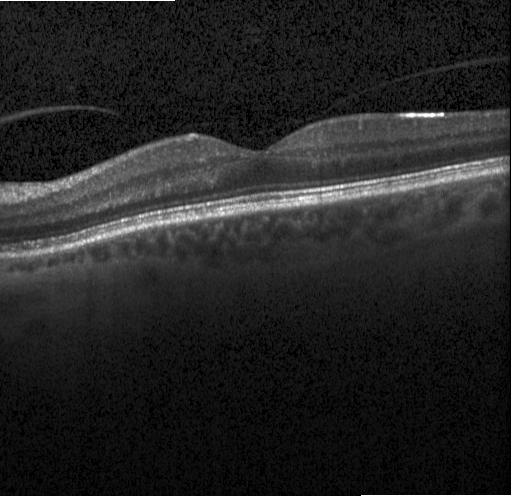
Retinal OCT cross-section showing no choroidal neovascularization, no diabetic macular edema, and no drusen.